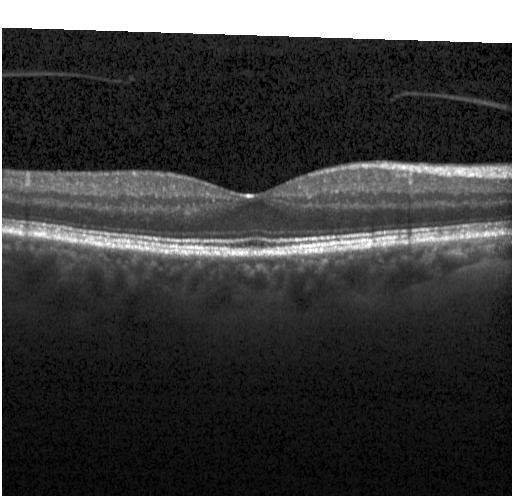 Diagnosis: no evidence of choroidal neovascularization, diabetic macular edema, or drusen.